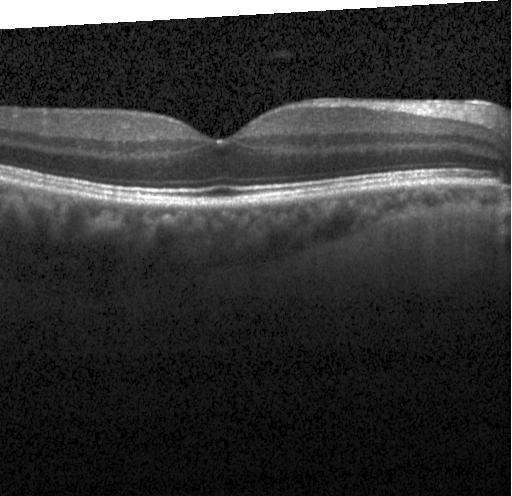
OCT line scan, spectral-domain OCT — Impression: no CNV, DME, or drusen.